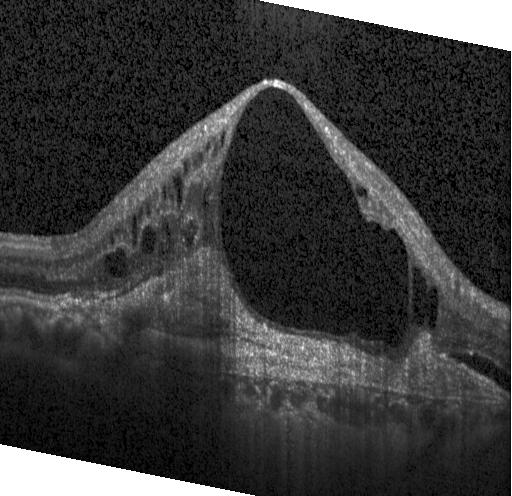

Retinal OCT B-scan; spectral-domain OCT; fovea-centered; instrument: Heidelberg Spectralis.
Diagnosis: a choroidal neovascular membrane.